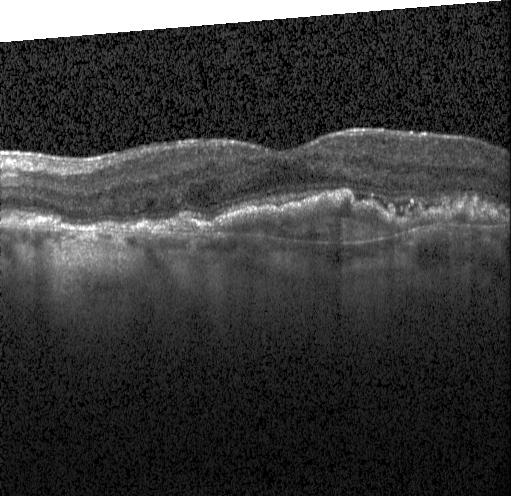
The scan shows choroidal neovascularization.